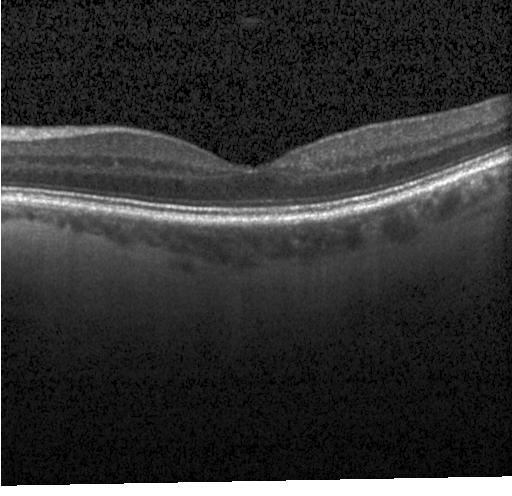

Macular scan, instrument: Heidelberg Spectralis, SD-OCT, optical coherence tomography B-scan.
This B-scan demonstrates no choroidal neovascularization, diabetic macular edema, or drusen.